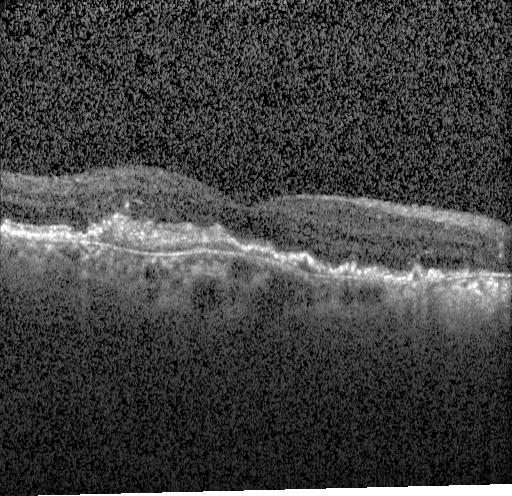
OCT B-scan showing choroidal neovascularization.